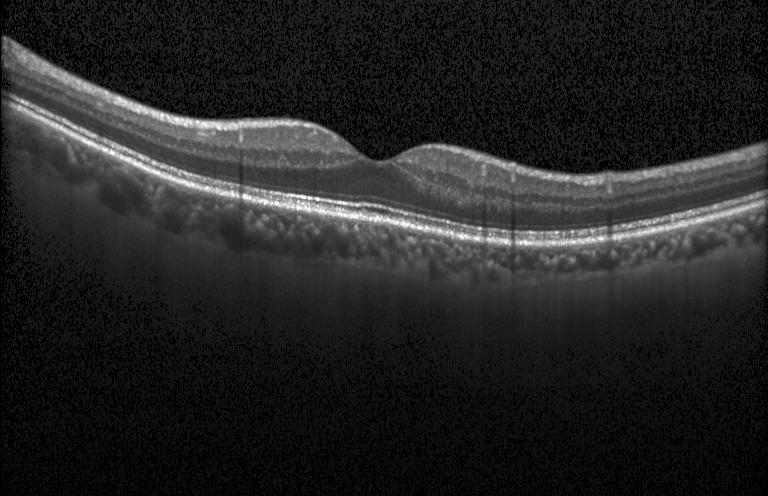
Heidelberg Spectralis OCT system. Spectral-domain optical coherence tomography. OCT B-scan — Diagnosis: no evidence of choroidal neovascularization, diabetic macular edema, or drusen.